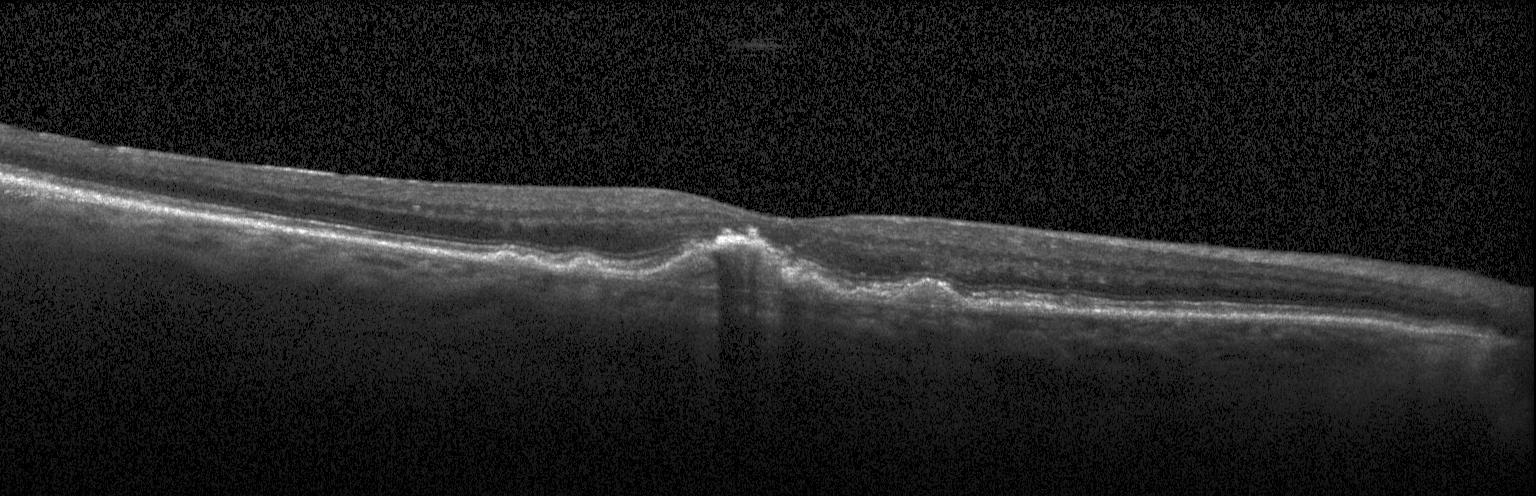 Optical coherence tomography scan, SD-OCT — Impression: choroidal neovascularization (CNV).